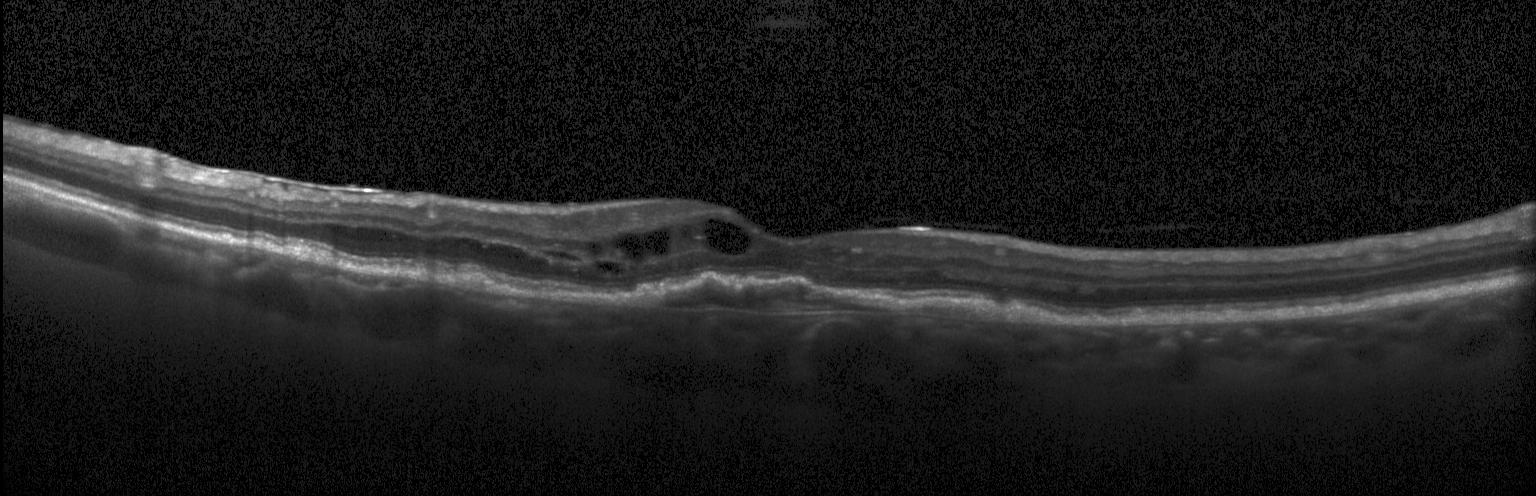 Macular scan; instrument: Heidelberg Spectralis; optical coherence tomography B-scan — Finding: CNV.